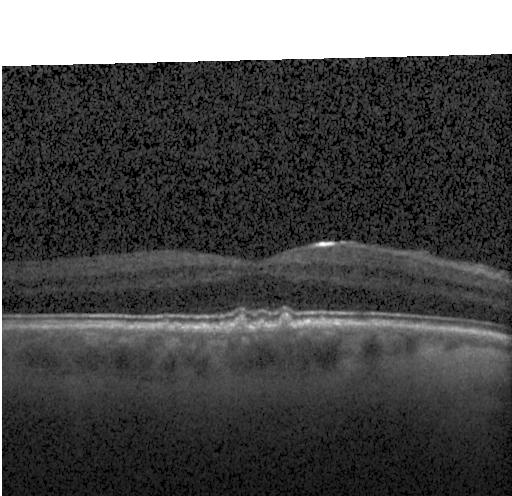
OCT B-scan showing sub-RPE drusenoid deposits.